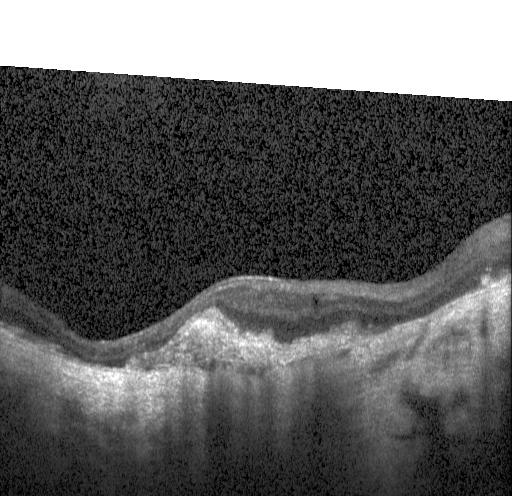

Impression: a choroidal neovascular membrane.